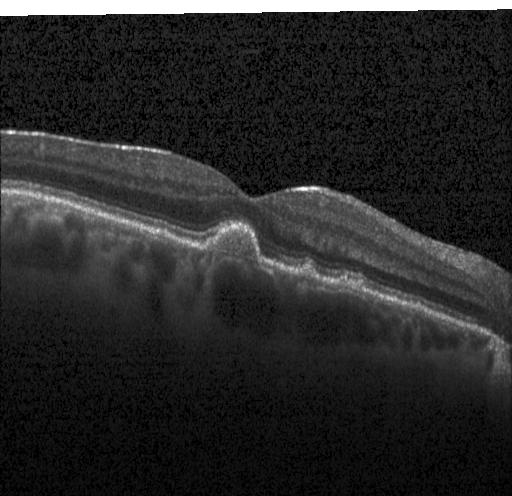 Spectral-domain optical coherence tomography. Macular scan. Instrument: Heidelberg Spectralis. OCT line scan. Sub-RPE drusenoid deposits.